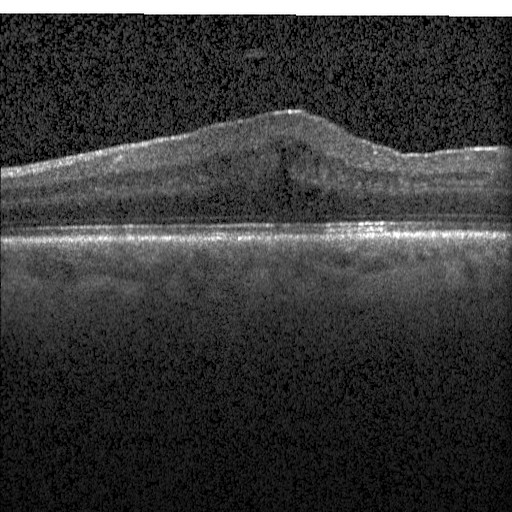 OCT line scan.
Impression: diabetic macular edema.